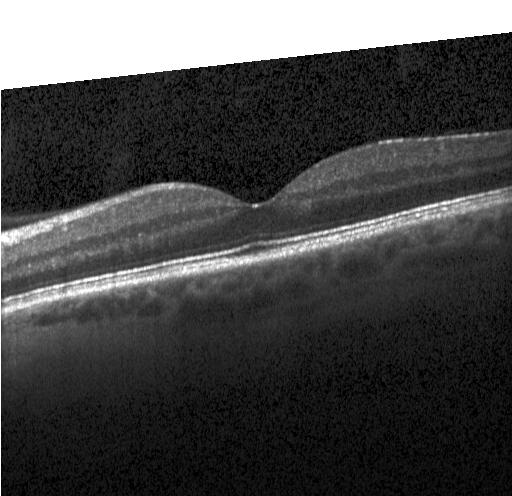 Macular OCT: no choroidal neovascularization, no diabetic macular edema, and no drusen.